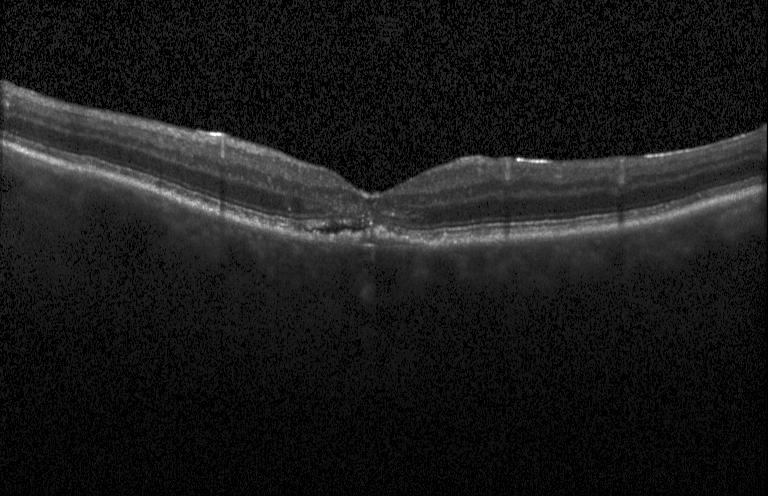 OCT line scan. Diagnosis: a choroidal neovascular membrane.